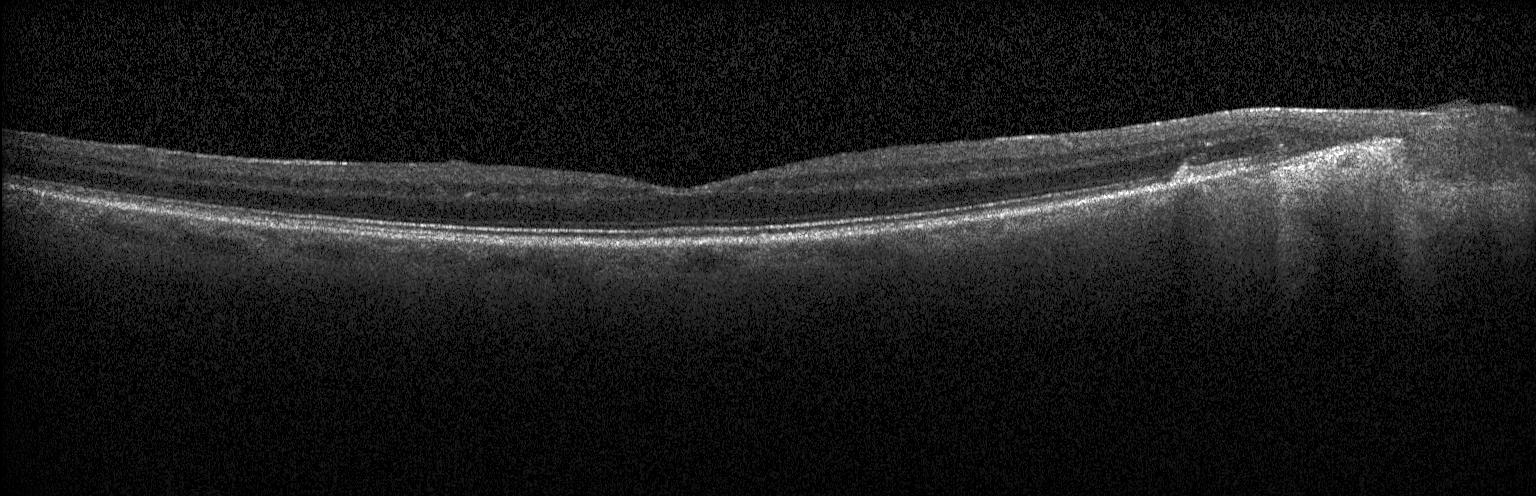

Diagnosis: no CNV, no DME, and no drusen.